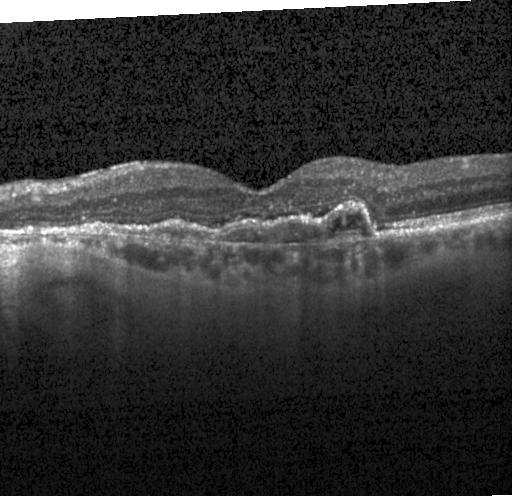 Retinal OCT cross-section
CNV.